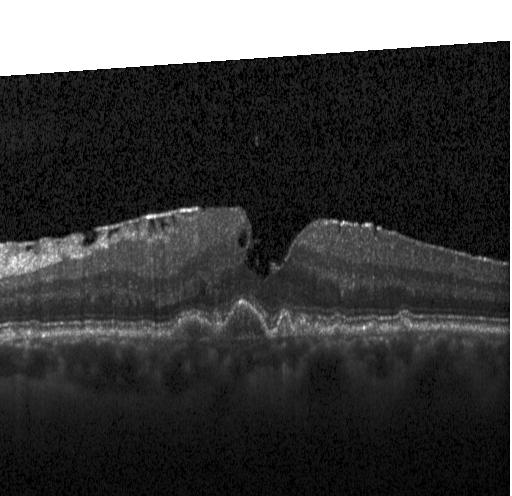
Macular OCT: CNV.